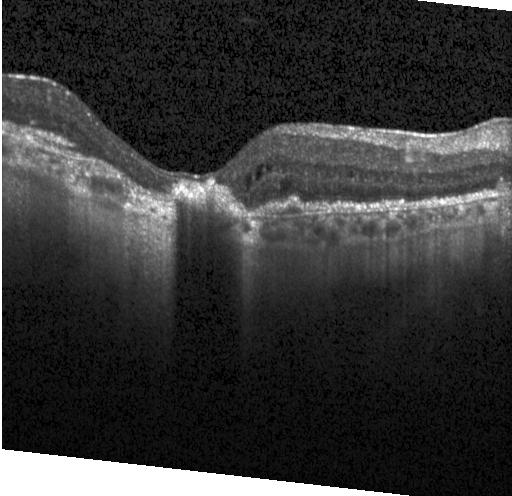
OCT scan showing a choroidal neovascular membrane.